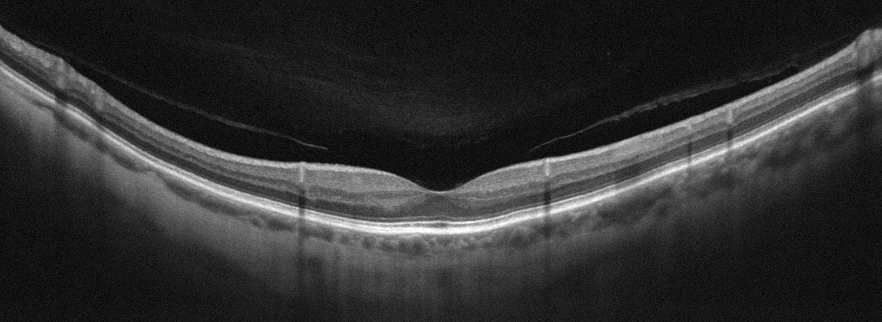 This B-scan demonstrates no AMD, DME, ERM, RAO, RVO, or VID.